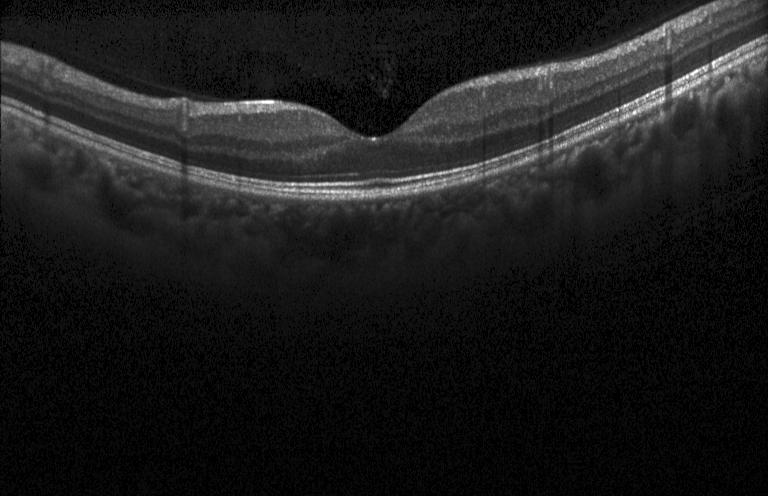

Heidelberg Spectralis OCT system. Horizontal scan through the fovea. OCT line scan.
No CNV, DME, or drusen.